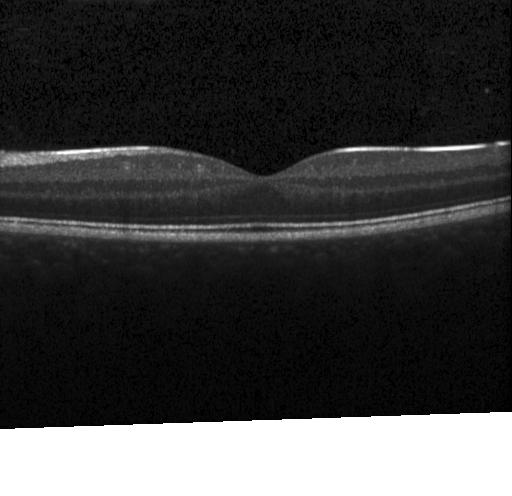
OCT B-scan — Assessment: no choroidal neovascularization, no diabetic macular edema, and no drusen.